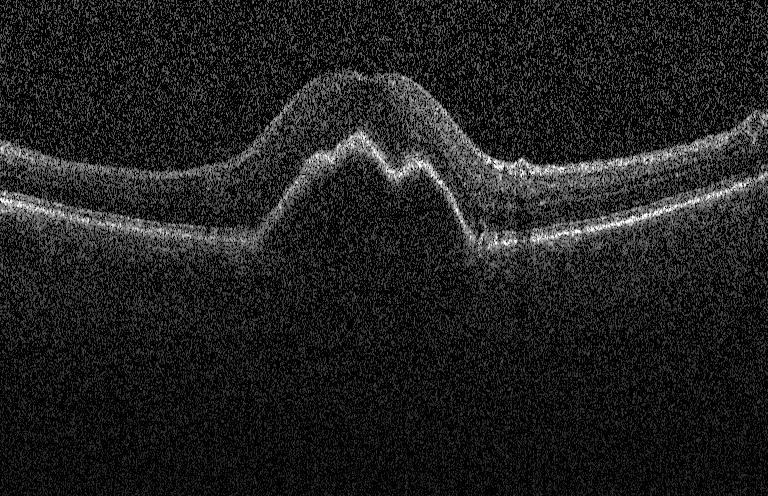 Spectral-domain OCT; retinal OCT B-scan; macular scan; instrument: Heidelberg Spectralis — OCT finding: choroidal neovascularization (CNV).